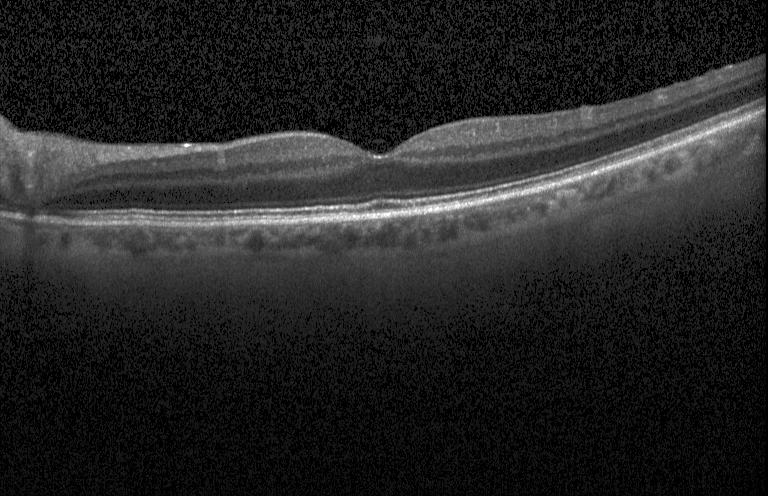
The scan shows no CNV, DME, or drusen.